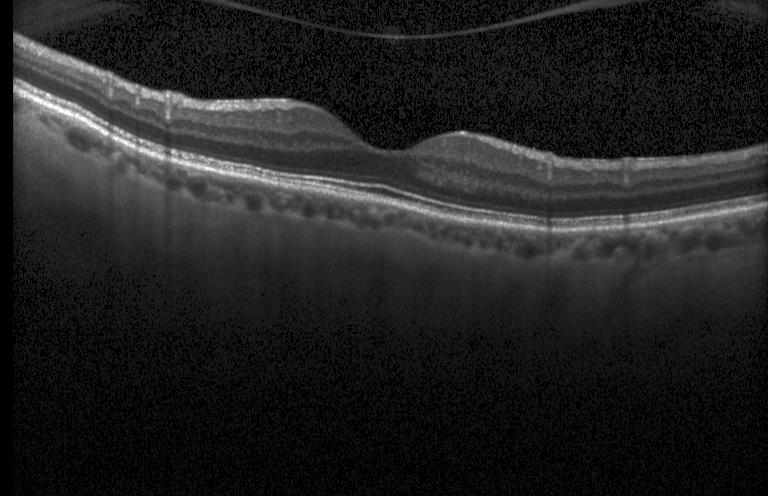 Optical coherence tomography B-scan; Heidelberg Spectralis OCT system
Diagnosis: no evidence of CNV, DME, or drusen.